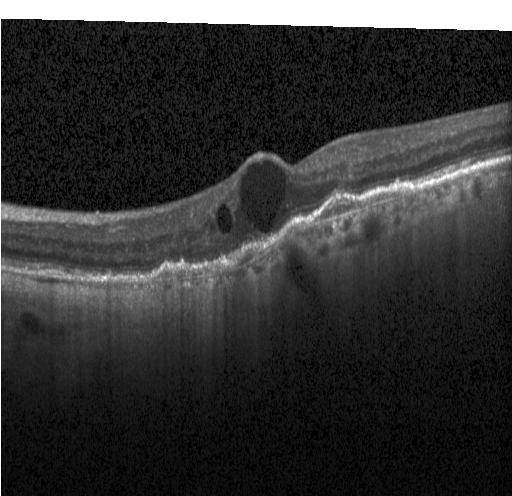

Heidelberg Spectralis OCT system; OCT line scan; spectral-domain optical coherence tomography; through the macula — Impression: a choroidal neovascular membrane.